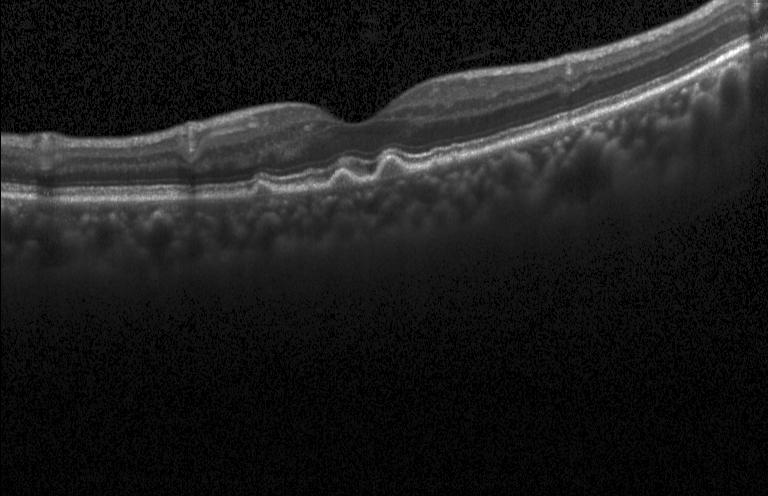 OCT B-scan, Heidelberg Spectralis OCT system, horizontal scan through the fovea
Impression: drusen.